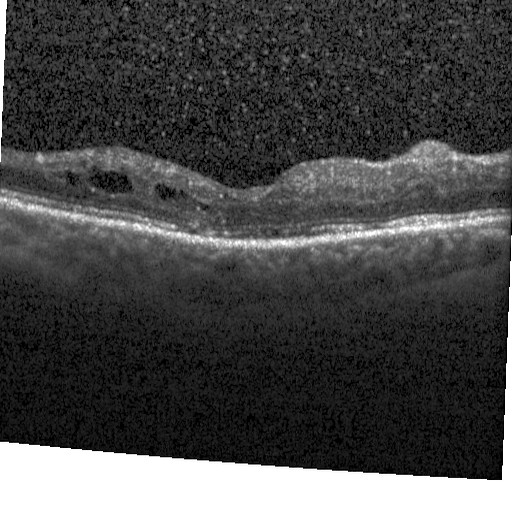 Retinal OCT cross-section · macular scan · Heidelberg Spectralis · spectral-domain optical coherence tomography.
Diabetic macular edema (DME).